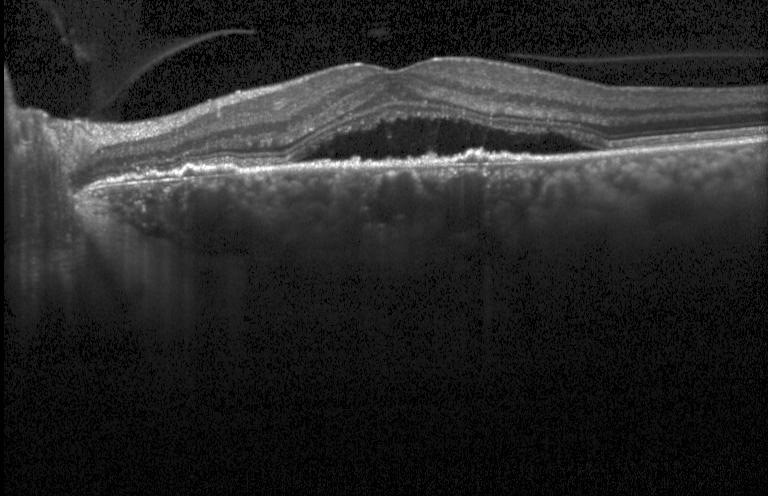
Retinal OCT B-scan.
Assessment: a choroidal neovascular membrane.